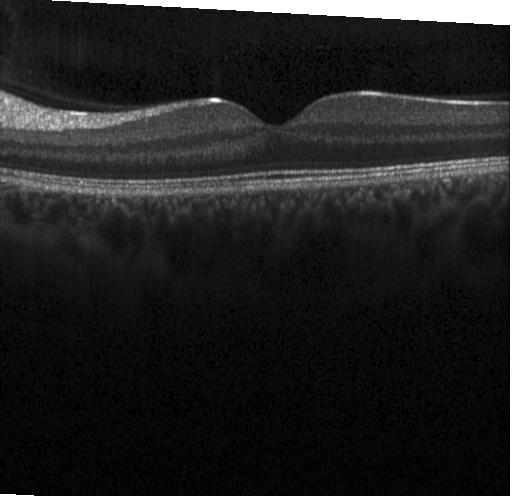 OCT finding: no evidence of CNV, DME, or drusen.